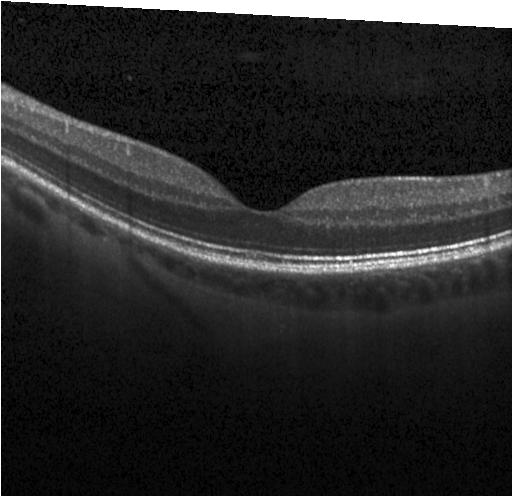
OCT B-scan, Heidelberg Spectralis.
Finding: neither choroidal neovascularization, diabetic macular edema, nor drusen.